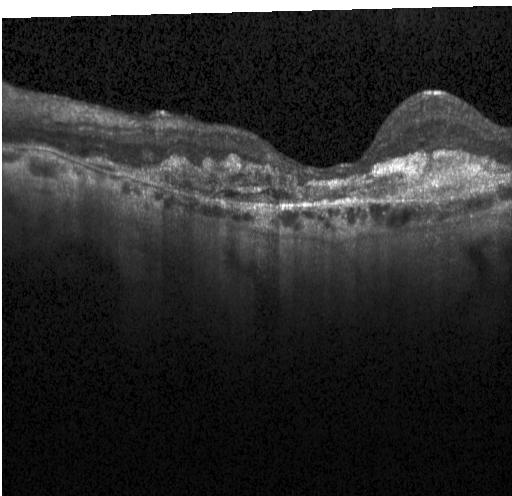

Fovea-centered · OCT B-scan.
Macular OCT: CNV.